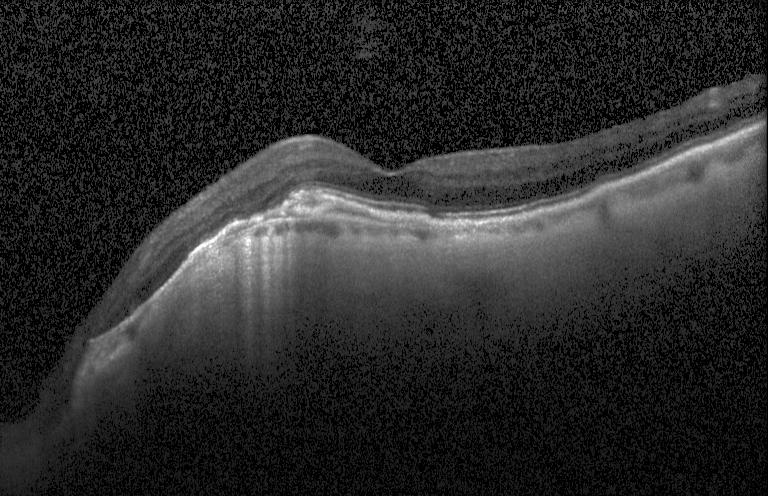

Through the macula; OCT B-scan; Heidelberg Spectralis OCT system; spectral-domain optical coherence tomography
Diagnosis: choroidal neovascularization.